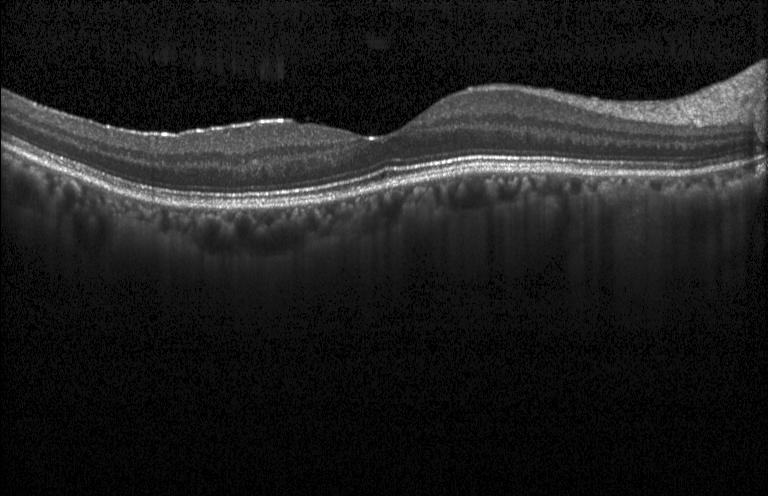 Macular scan. Retinal OCT B-scan. Diagnosis: no choroidal neovascularization, no diabetic macular edema, and no drusen.